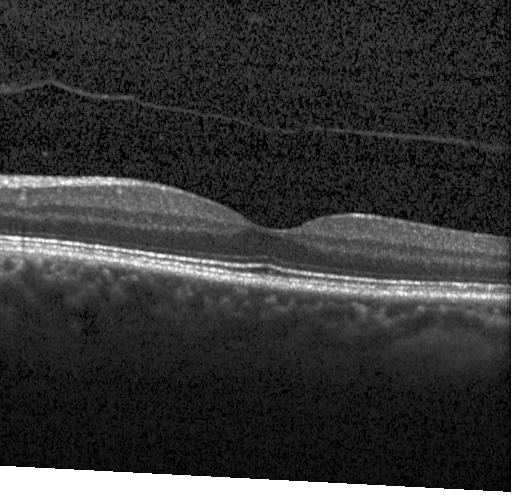
Retinal OCT B-scan.
Impression: no evidence of CNV, DME, or drusen.